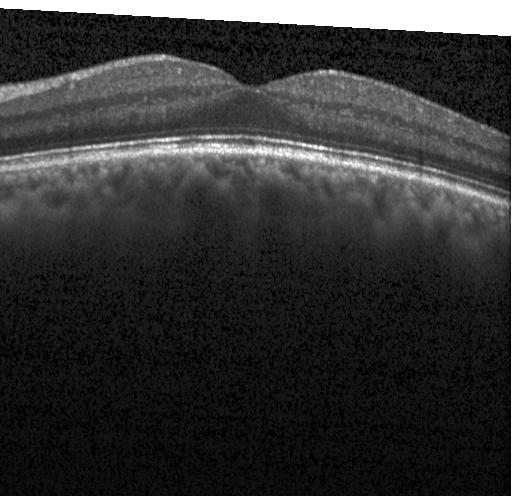

Acquired on a Heidelberg Spectralis; spectral-domain OCT; optical coherence tomography B-scan
Assessment: neither choroidal neovascularization, diabetic macular edema, nor drusen.